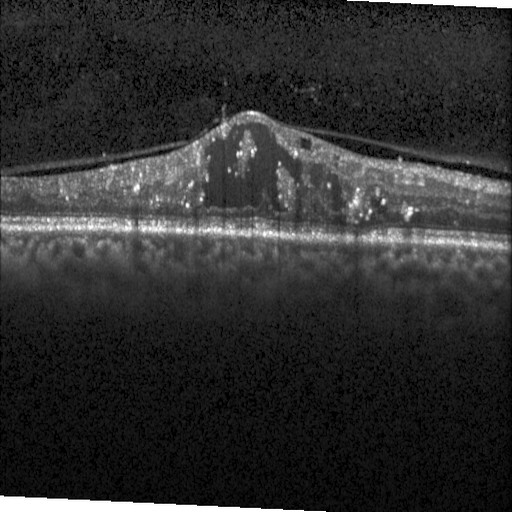
Macular OCT: diabetic macular edema (DME).